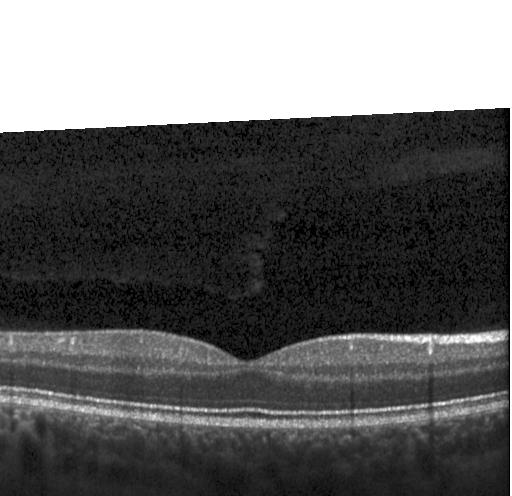 Optical coherence tomography scan
Impression: no choroidal neovascularization, no diabetic macular edema, and no drusen.